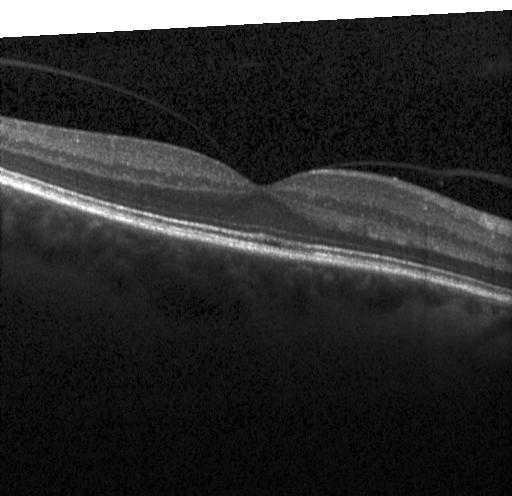

Impression: no choroidal neovascularization, no diabetic macular edema, and no drusen.